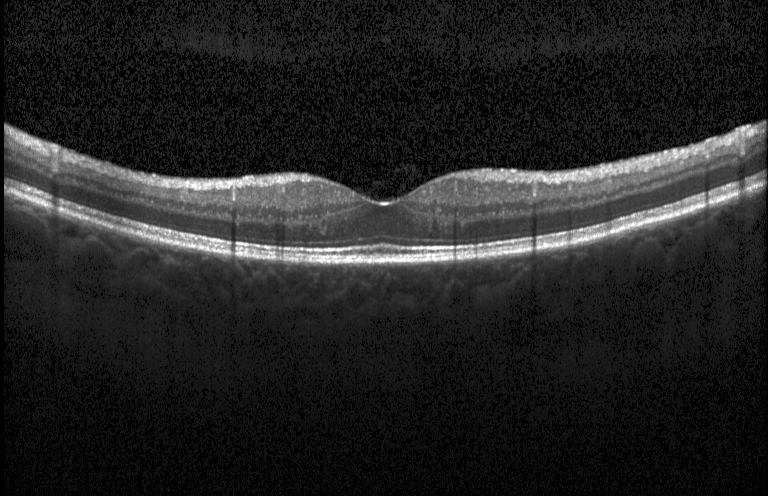
Retinal OCT B-scan, macular scan, Heidelberg Spectralis OCT system
Diagnosis: neither choroidal neovascularization, diabetic macular edema, nor drusen.